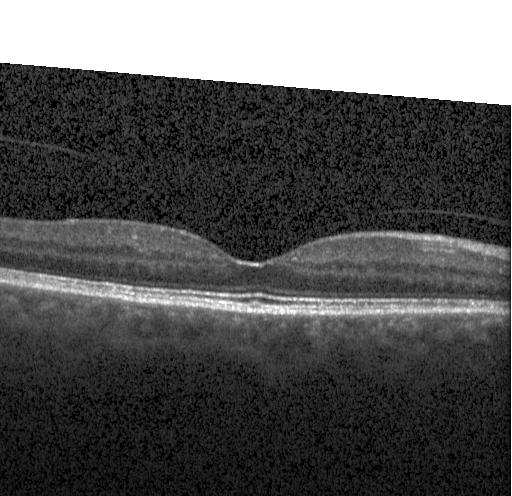

Impression: no evidence of CNV, DME, or drusen.